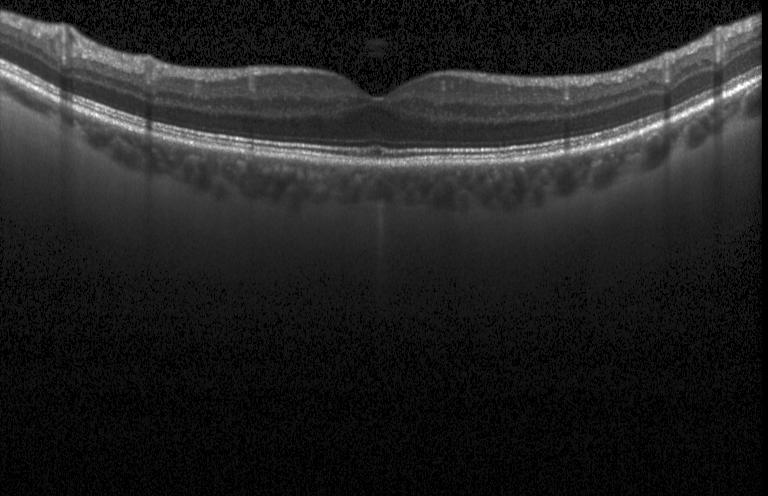 OCT B-scan
Dx: no evidence of CNV, DME, or drusen.